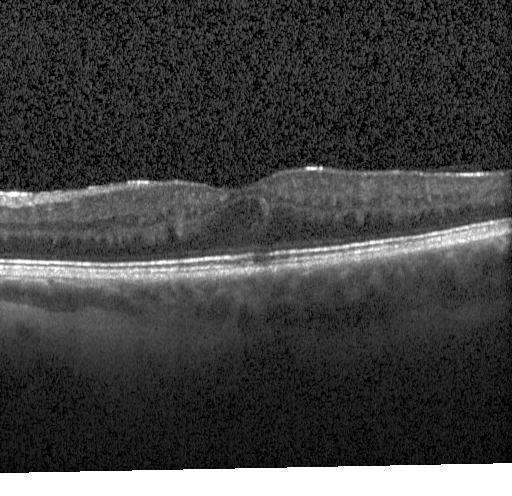 Spectral-domain OCT B-scan: no CNV, no DME, and no drusen.